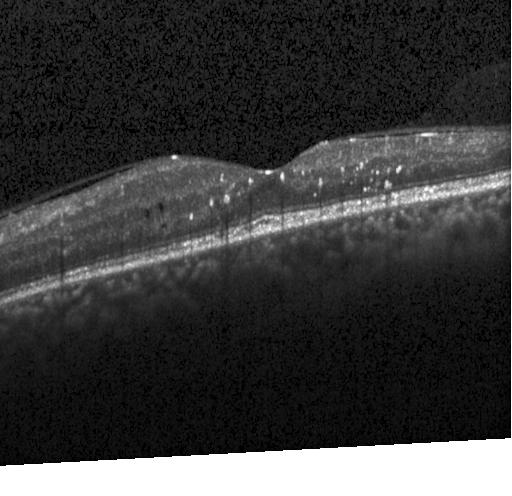

Heidelberg Spectralis. Macular scan. Spectral-domain optical coherence tomography. Retinal OCT cross-section.
Impression: DME.